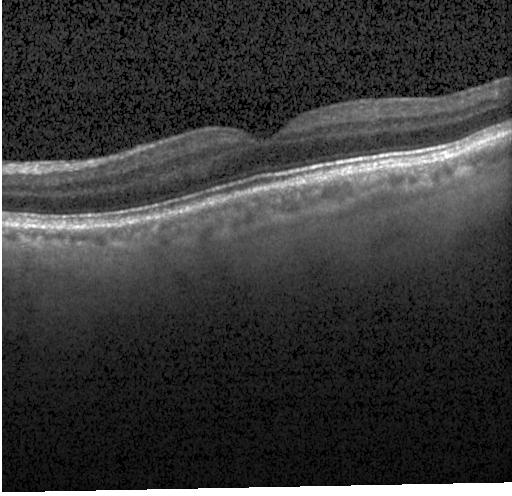

Acquired on a Heidelberg Spectralis; through the macula; retinal OCT B-scan; spectral-domain OCT
Finding: no evidence of choroidal neovascularization, diabetic macular edema, or drusen.